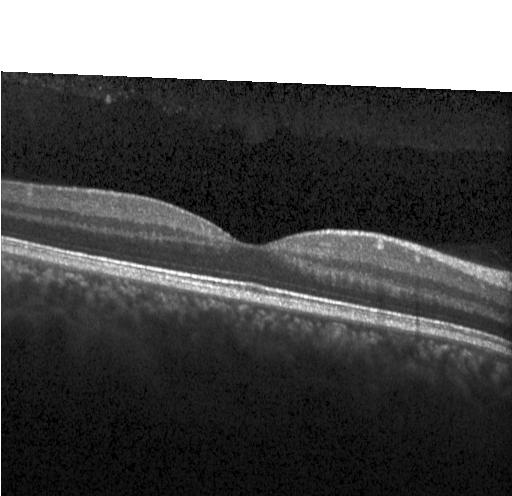

No evidence of choroidal neovascularization, diabetic macular edema, or drusen.